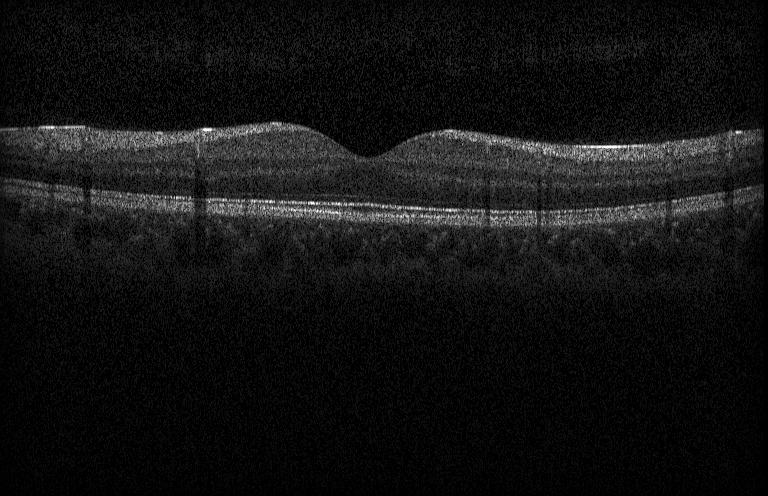
Macular OCT demonstrating no evidence of choroidal neovascularization, diabetic macular edema, or drusen.